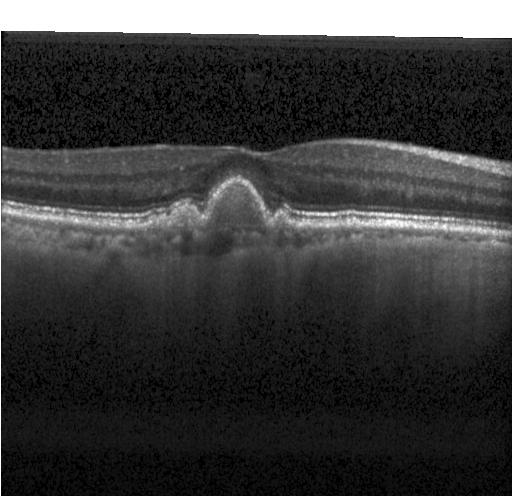 Optical coherence tomography B-scan.
Assessment: CNV.